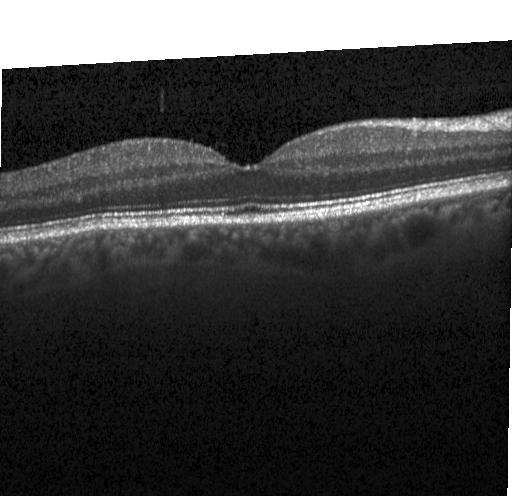
Diagnosis: no CNV, no DME, and no drusen.